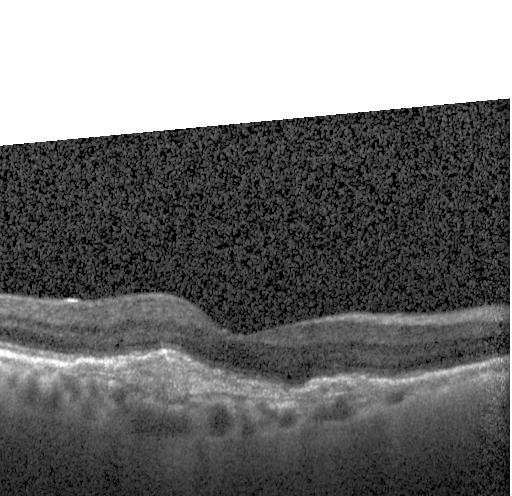 Through the macula. OCT line scan. SD-OCT.
This B-scan demonstrates CNV.